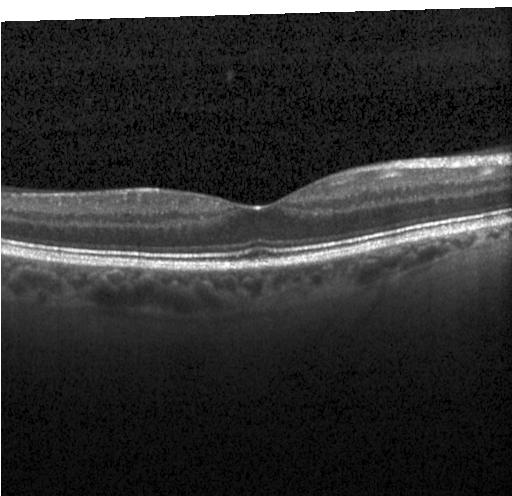
Heidelberg Spectralis. Spectral-domain OCT. Macular scan. OCT line scan
OCT finding: neither CNV, DME, nor drusen.